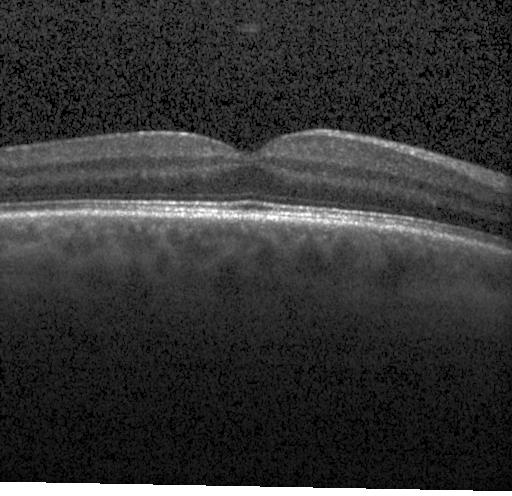

Diagnosis: neither choroidal neovascularization, diabetic macular edema, nor drusen.